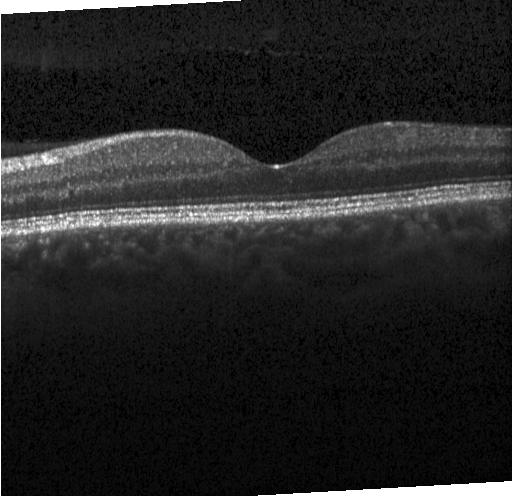
OCT scan showing no evidence of choroidal neovascularization, diabetic macular edema, or drusen.